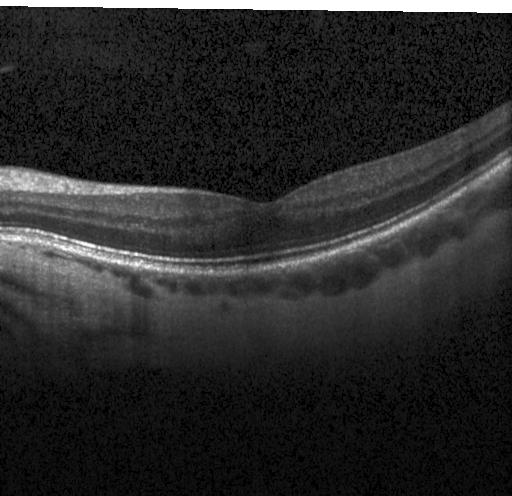 Dx: no CNV, DME, or drusen.